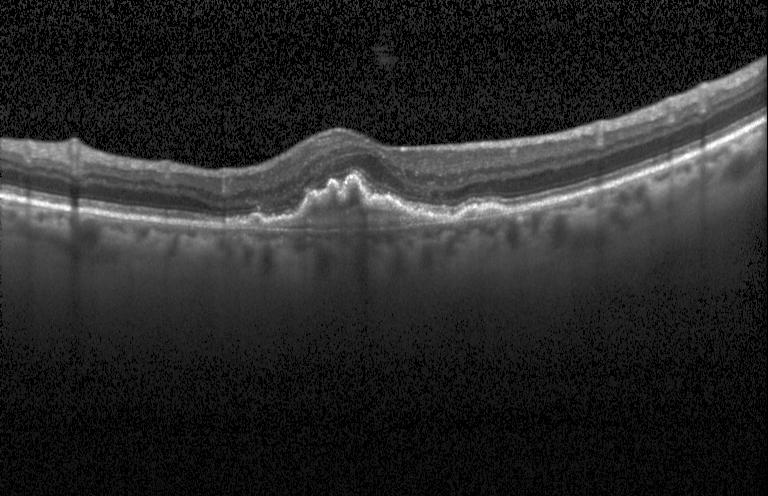
Through the macula · acquired on a Heidelberg Spectralis · optical coherence tomography scan
Finding: choroidal neovascularization.